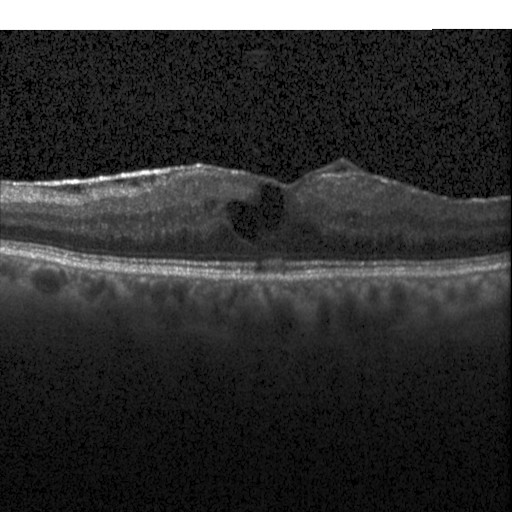 OCT B-scan showing diabetic macular edema (DME).